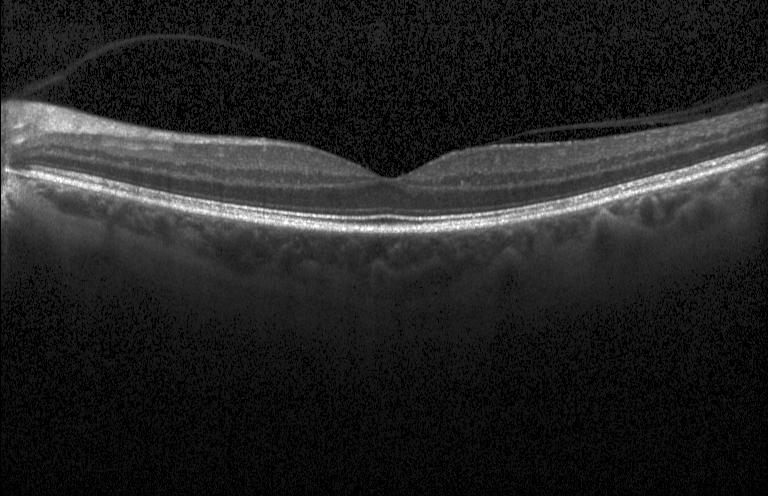 OCT B-scan showing neither choroidal neovascularization, diabetic macular edema, nor drusen.